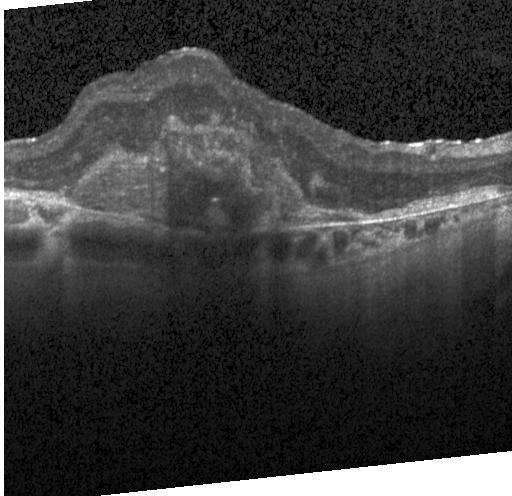

Diagnosis: a choroidal neovascular membrane.